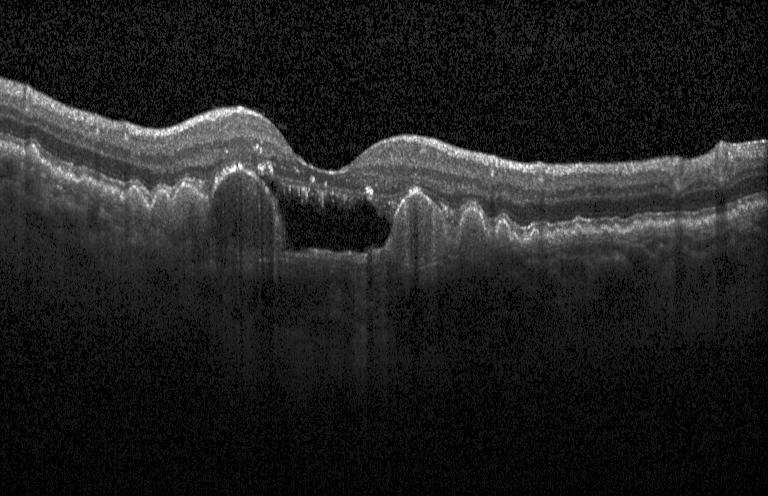
Impression: a choroidal neovascular membrane.